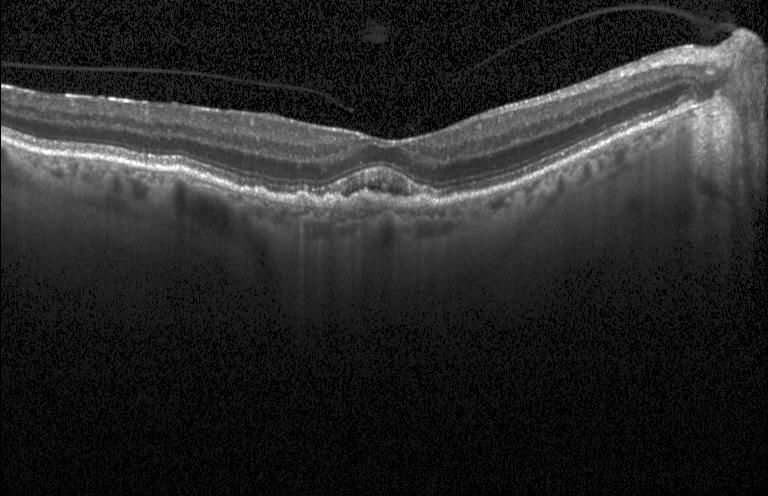 OCT B-scan. Spectral-domain optical coherence tomography. Instrument: Heidelberg Spectralis.
Impression: CNV.